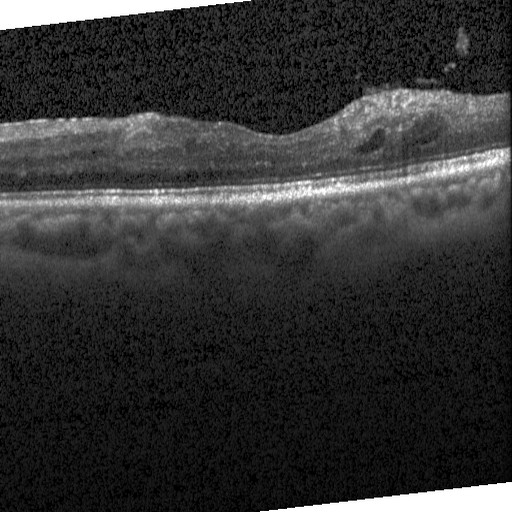

OCT finding: diabetic macular edema (DME).